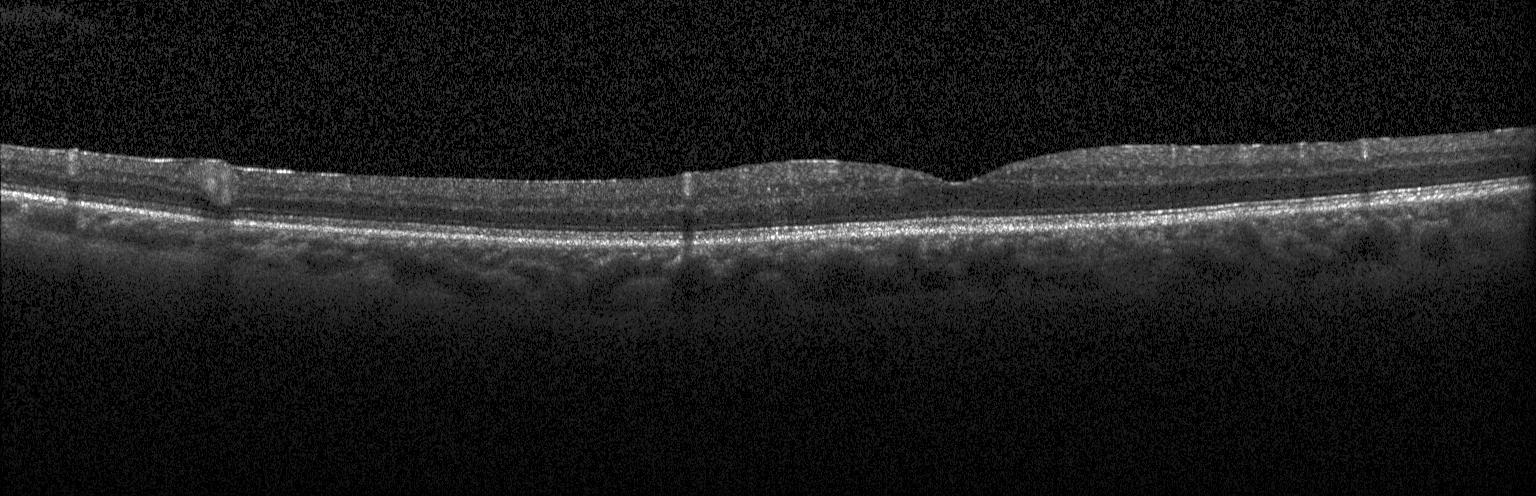 Macular scan · spectral-domain optical coherence tomography · optical coherence tomography scan · acquired on a Heidelberg Spectralis.
Assessment: no choroidal neovascularization, no diabetic macular edema, and no drusen.